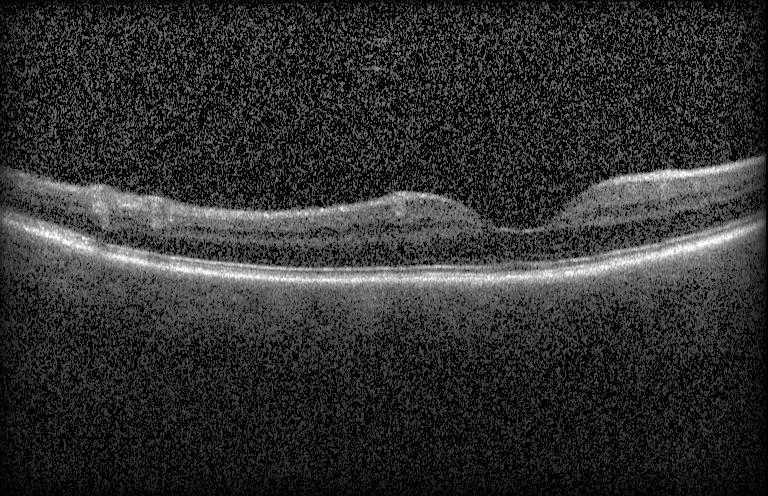

OCT B-scan; spectral-domain optical coherence tomography.
Finding: no evidence of choroidal neovascularization, diabetic macular edema, or drusen.